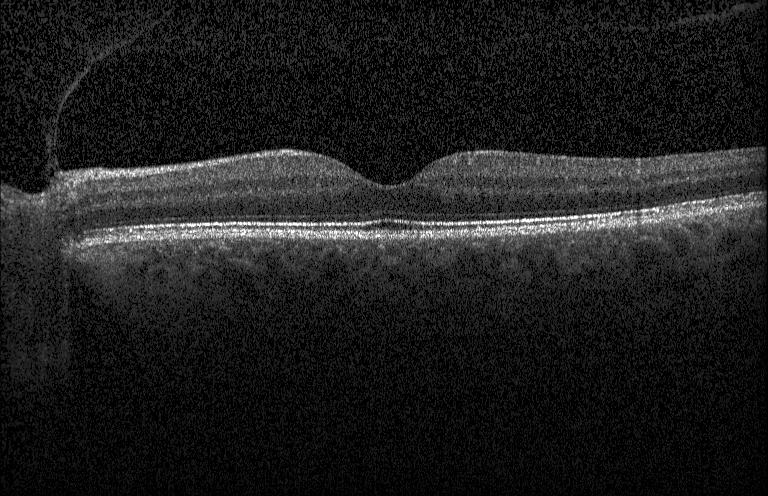
Impression: neither choroidal neovascularization, diabetic macular edema, nor drusen.